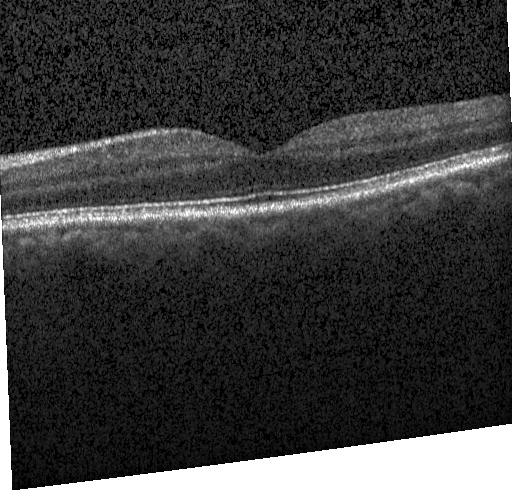
Optical coherence tomography scan; macular scan; instrument: Heidelberg Spectralis; spectral-domain optical coherence tomography. Diagnosis: neither choroidal neovascularization, diabetic macular edema, nor drusen.